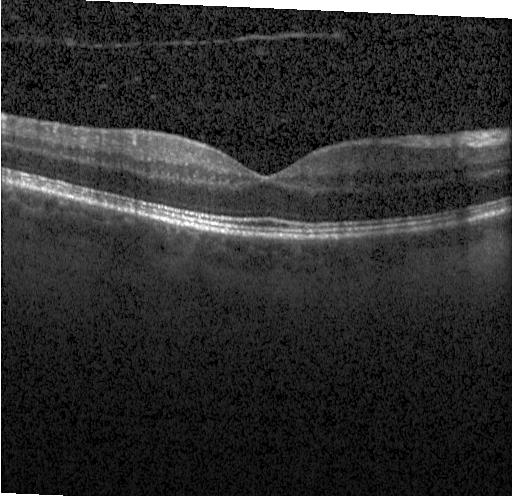
Retinal OCT cross-section.
The scan shows no choroidal neovascularization, diabetic macular edema, or drusen.